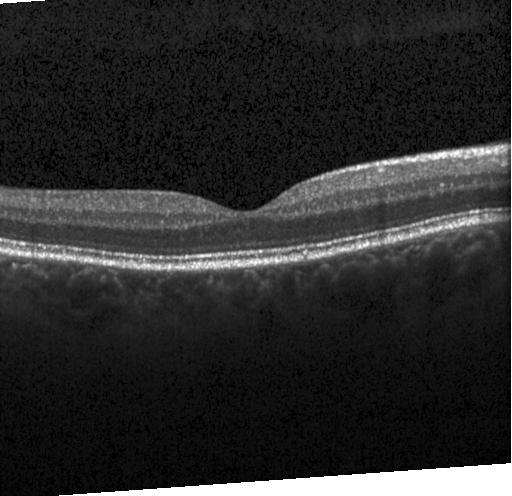
Diagnosis: neither CNV, DME, nor drusen.